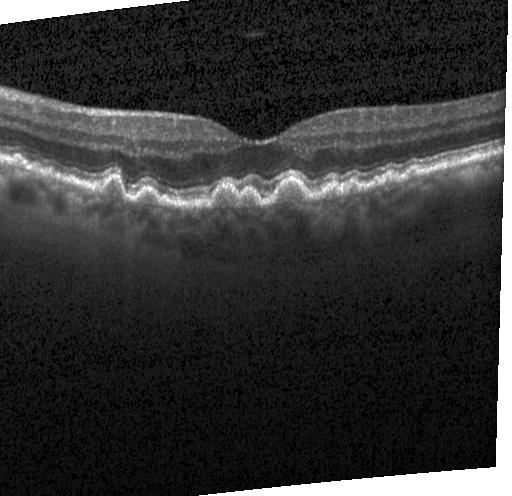
Impression: multiple drusen.